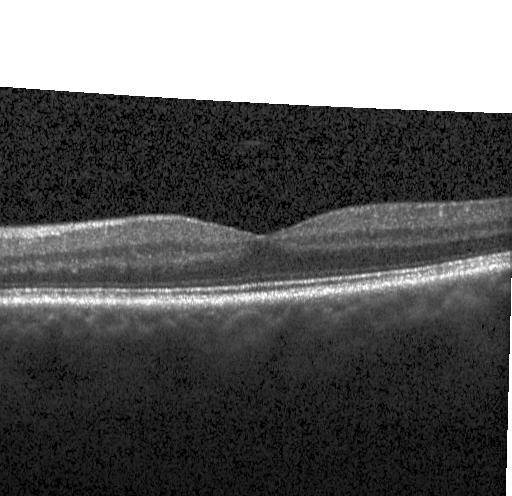 OCT B-scan showing no CNV, DME, or drusen.